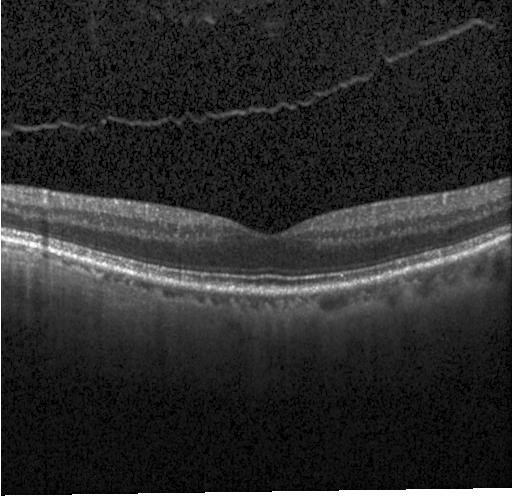
SD-OCT · retinal OCT B-scan — Finding: no evidence of CNV, DME, or drusen.